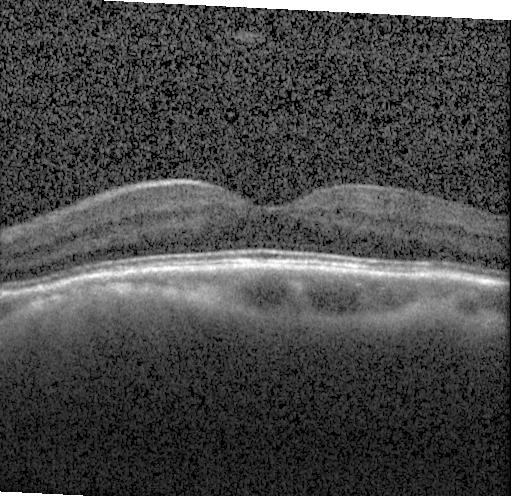
Diagnosis: neither CNV, DME, nor drusen.